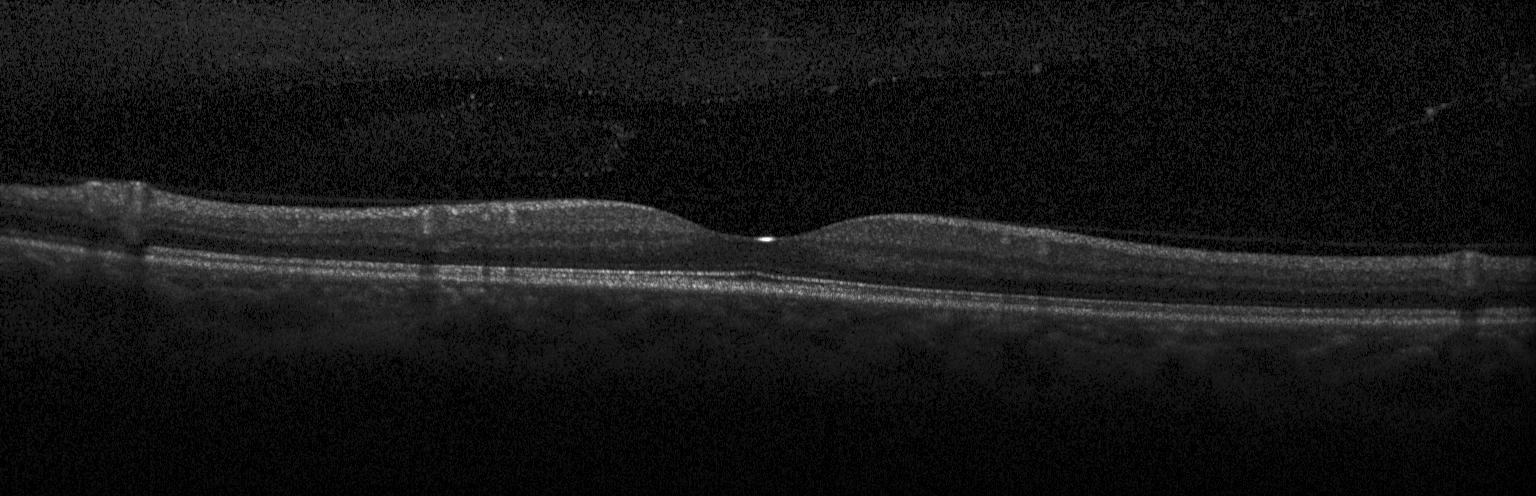
Impression: no choroidal neovascularization, diabetic macular edema, or drusen.